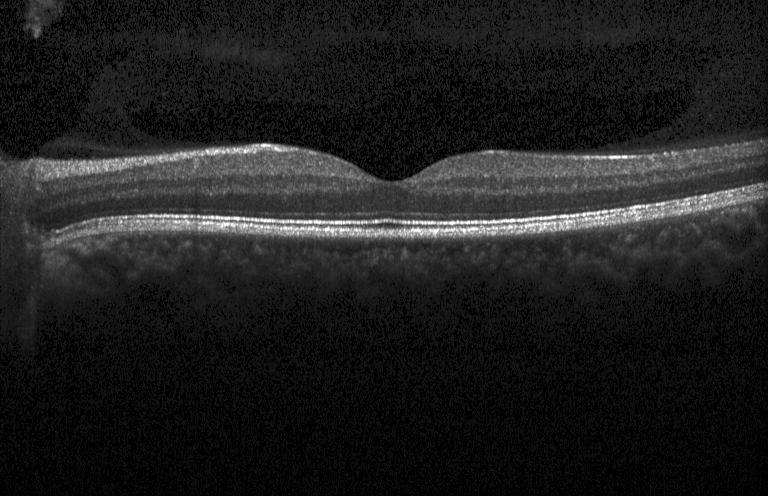 Retinal OCT B-scan. Diagnosis: neither choroidal neovascularization, diabetic macular edema, nor drusen.